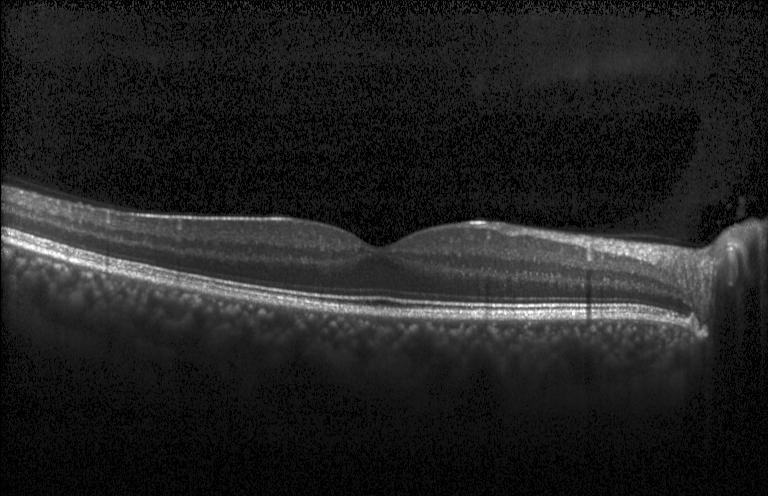

Heidelberg Spectralis · fovea-centered · OCT line scan · spectral-domain OCT
Diagnosis: no evidence of choroidal neovascularization, diabetic macular edema, or drusen.